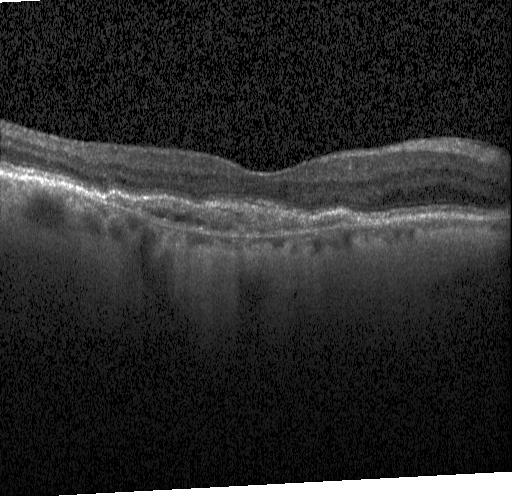
Impression: a choroidal neovascular membrane.